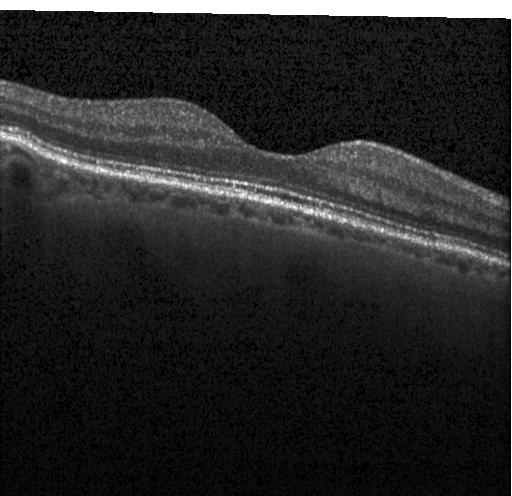
Through the macula · Heidelberg Spectralis · optical coherence tomography B-scan · spectral-domain OCT. Assessment: no CNV, DME, or drusen.